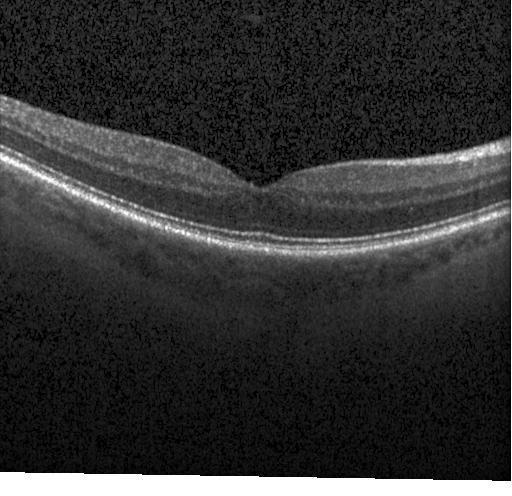 Diagnosis: no evidence of choroidal neovascularization, diabetic macular edema, or drusen.